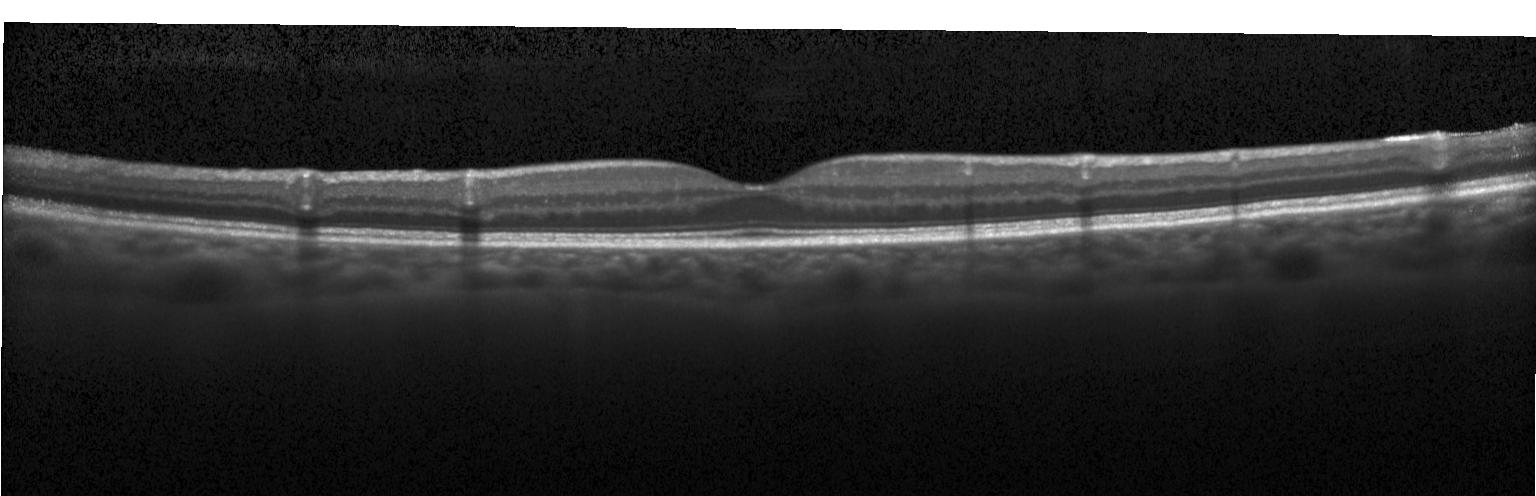
Diagnosis: no choroidal neovascularization, no diabetic macular edema, and no drusen.